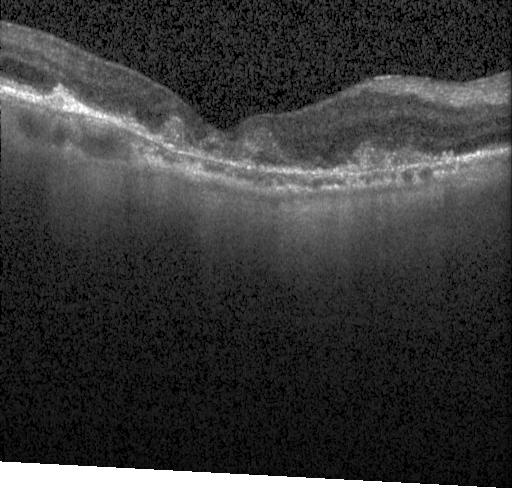 Through the macula. Instrument: Heidelberg Spectralis. Retinal OCT cross-section. Spectral-domain optical coherence tomography.
Impression: a choroidal neovascular membrane.